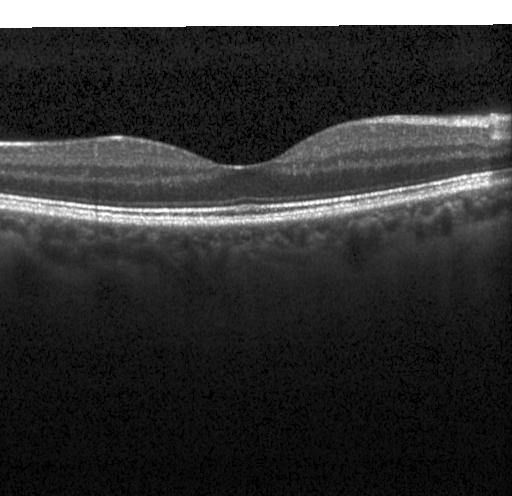
Optical coherence tomography scan, spectral-domain optical coherence tomography, acquired on a Heidelberg Spectralis, macular scan
Assessment: no evidence of choroidal neovascularization, diabetic macular edema, or drusen.